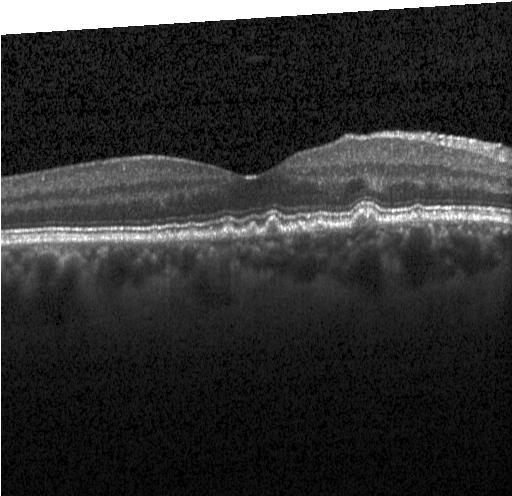 Optical coherence tomography B-scan, spectral-domain optical coherence tomography. Sub-RPE drusenoid deposits.